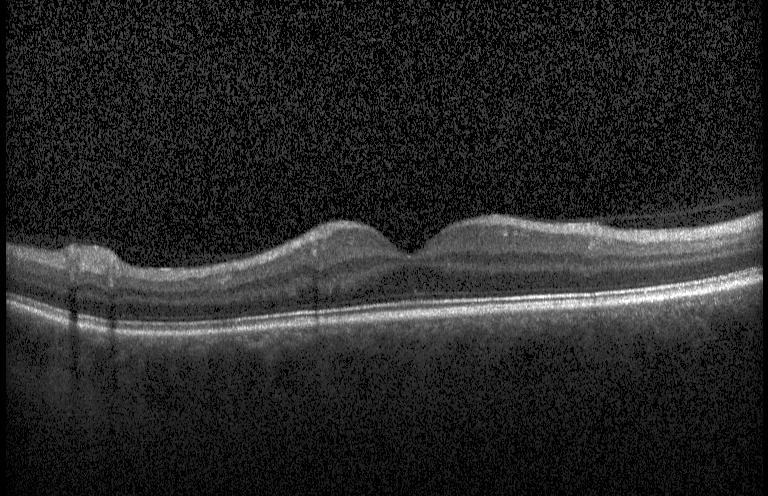 Impression: no choroidal neovascularization, no diabetic macular edema, and no drusen.